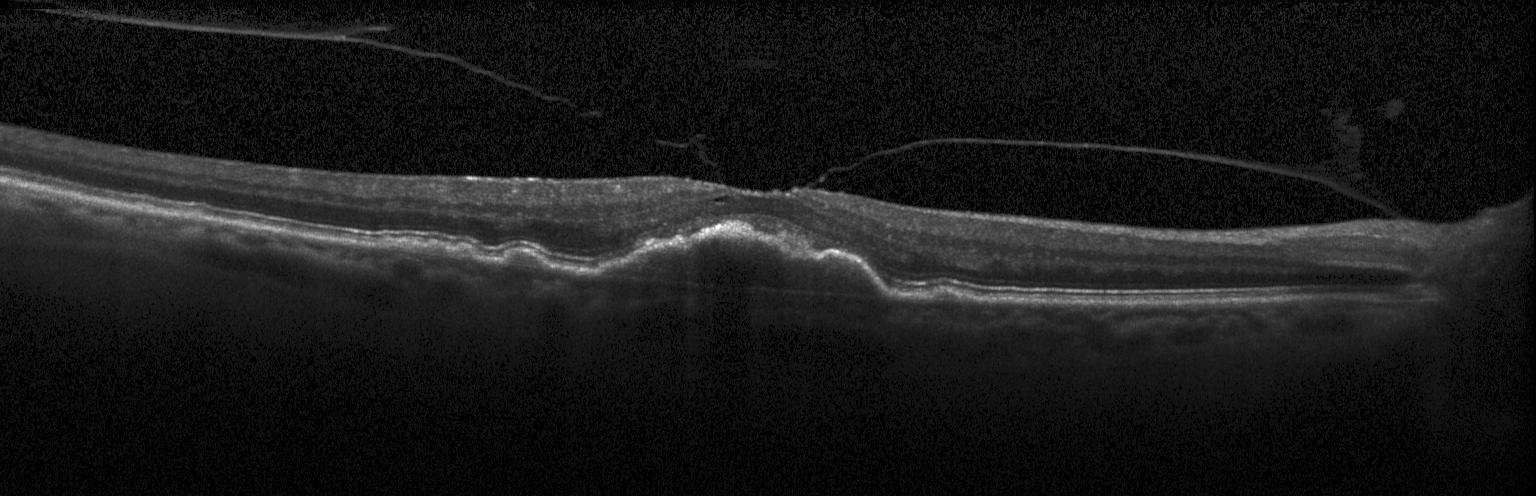 Retinal OCT cross-section. Macular scan. Instrument: Heidelberg Spectralis. Spectral-domain OCT. This B-scan demonstrates a choroidal neovascular membrane.